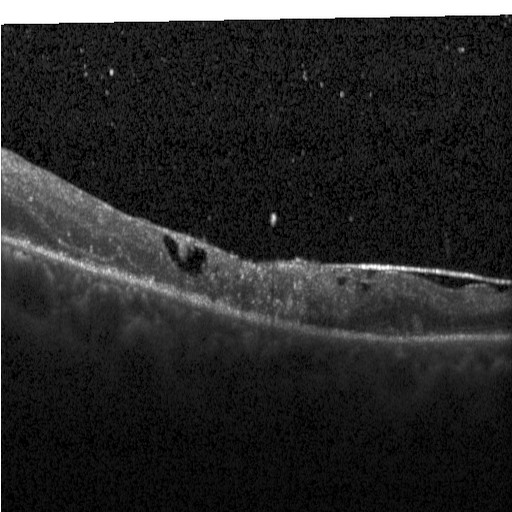

Impression: DME.